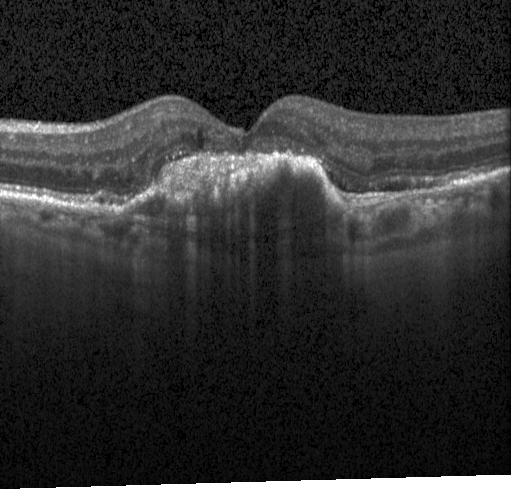 Optical coherence tomography B-scan — Macular OCT: a choroidal neovascular membrane.